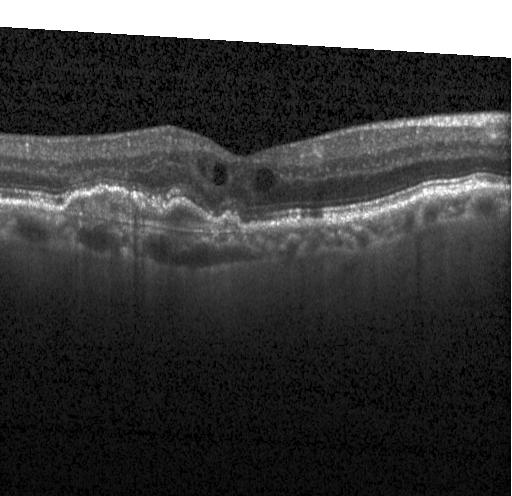
OCT scan showing CNV.